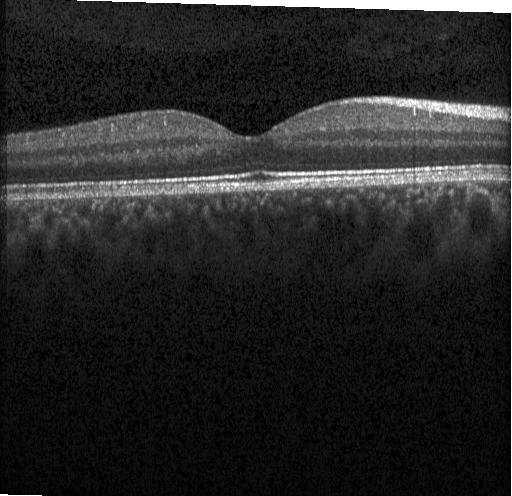
OCT B-scan.
Finding: no choroidal neovascularization, diabetic macular edema, or drusen.